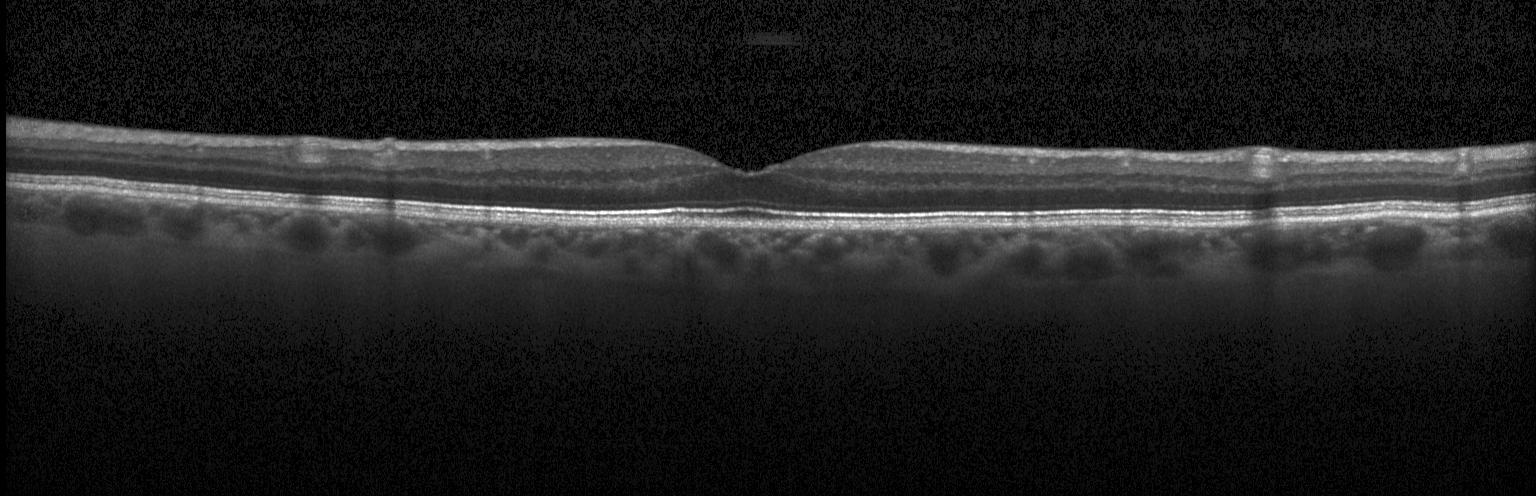
Acquired on a Heidelberg Spectralis · optical coherence tomography scan · centered on the fovea · spectral-domain optical coherence tomography
Diagnosis: neither choroidal neovascularization, diabetic macular edema, nor drusen.